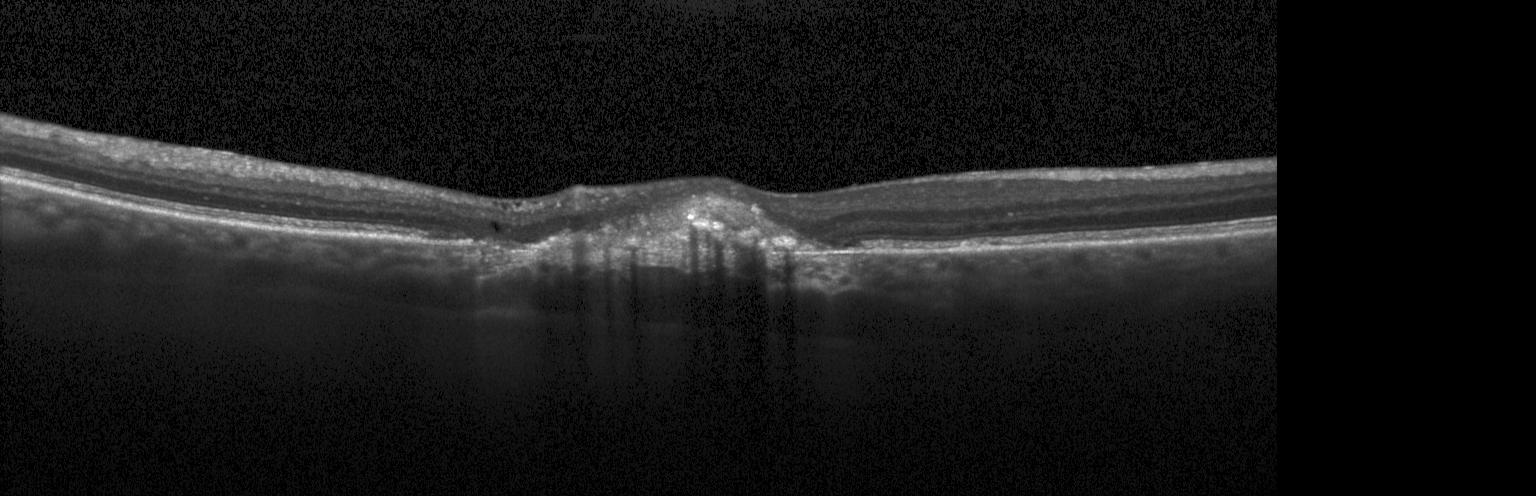

Assessment: a choroidal neovascular membrane.